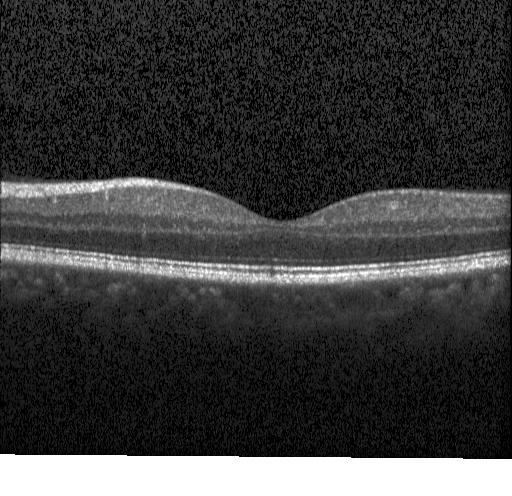

This B-scan demonstrates neither choroidal neovascularization, diabetic macular edema, nor drusen.